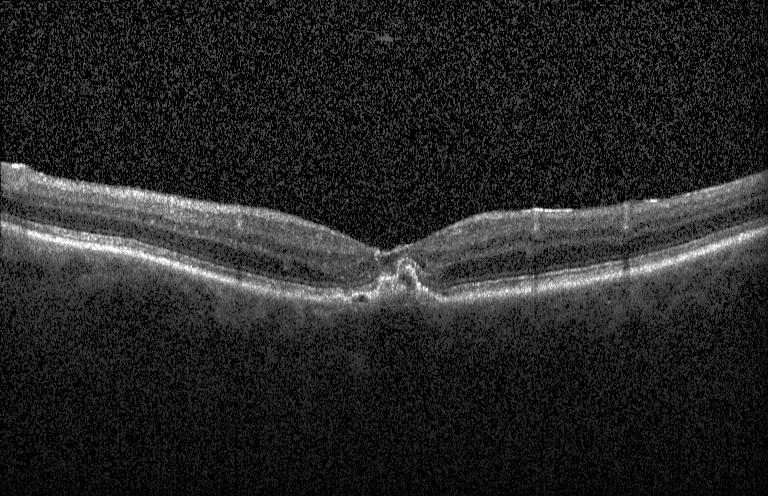

Retinal OCT B-scan; Heidelberg Spectralis OCT system; SD-OCT; fovea-centered
OCT finding: a choroidal neovascular membrane.